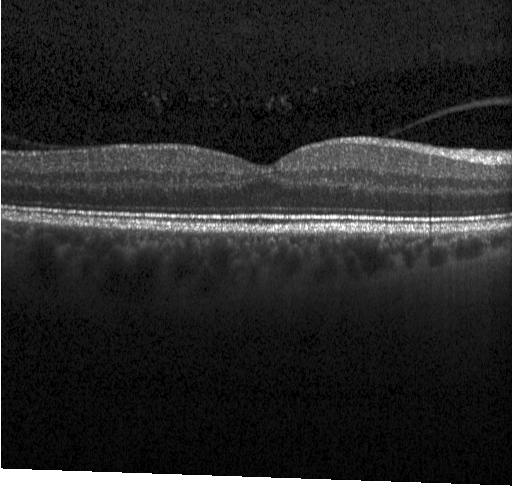

Heidelberg Spectralis · OCT B-scan · through the macula · SD-OCT — Macular OCT: no choroidal neovascularization, no diabetic macular edema, and no drusen.